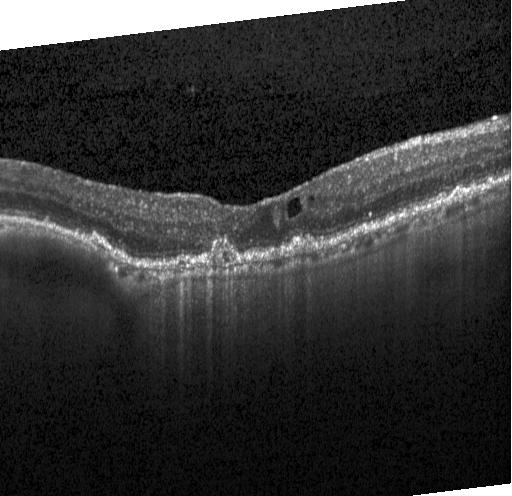 Dx: a choroidal neovascular membrane.